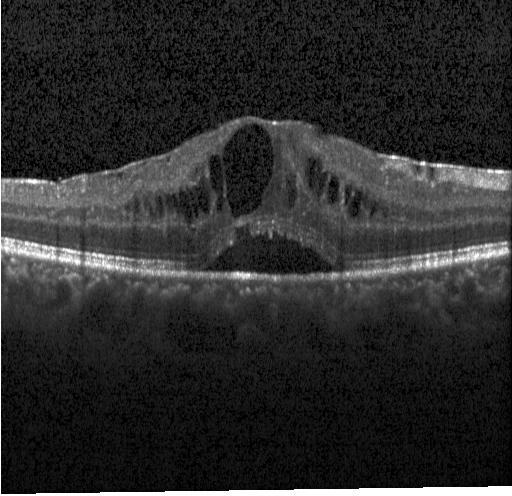
Spectral-domain optical coherence tomography · optical coherence tomography scan · Heidelberg Spectralis OCT system · macular scan
Finding: diabetic macular edema.